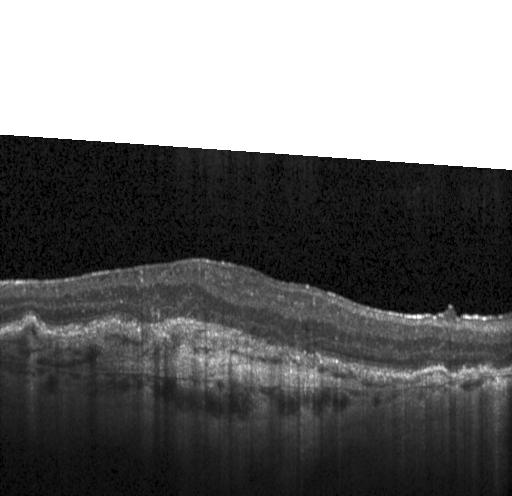 Macular scan. Optical coherence tomography scan. SD-OCT.
Impression: choroidal neovascularization.